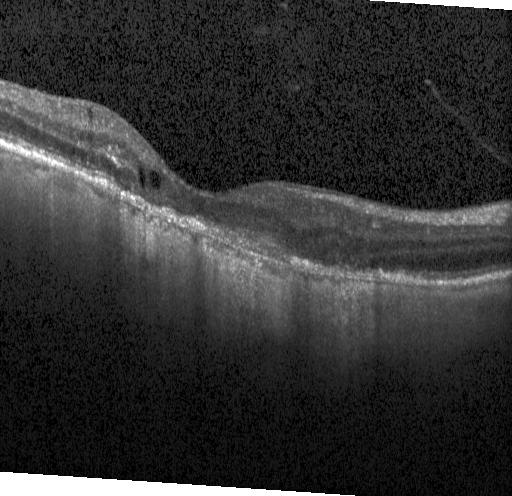 Diagnosis: a choroidal neovascular membrane.